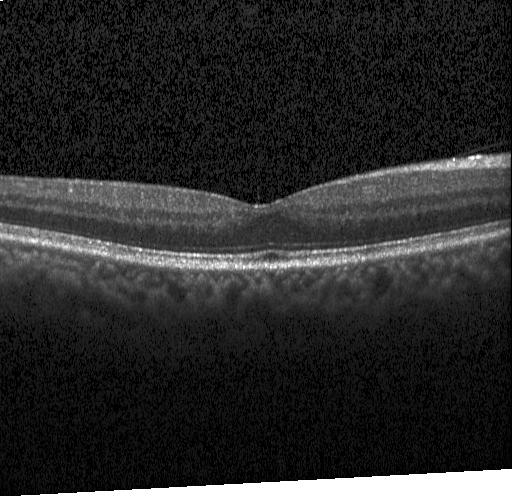 OCT finding: neither choroidal neovascularization, diabetic macular edema, nor drusen.